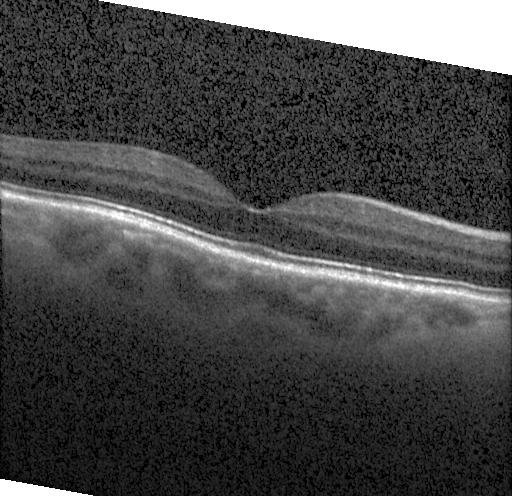

Spectral-domain OCT; Heidelberg Spectralis OCT system; retinal OCT cross-section.
Diagnosis: no evidence of choroidal neovascularization, diabetic macular edema, or drusen.